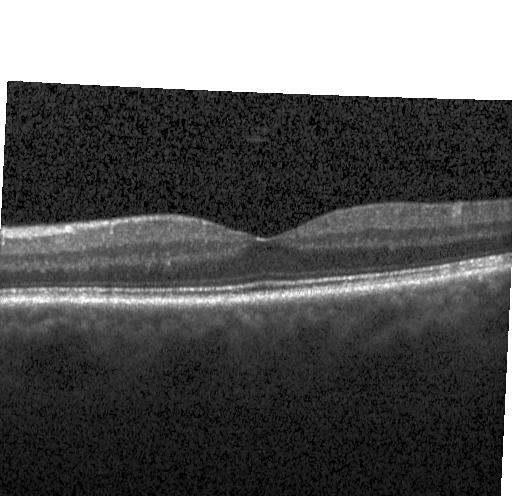 OCT line scan — Assessment: no CNV, no DME, and no drusen.